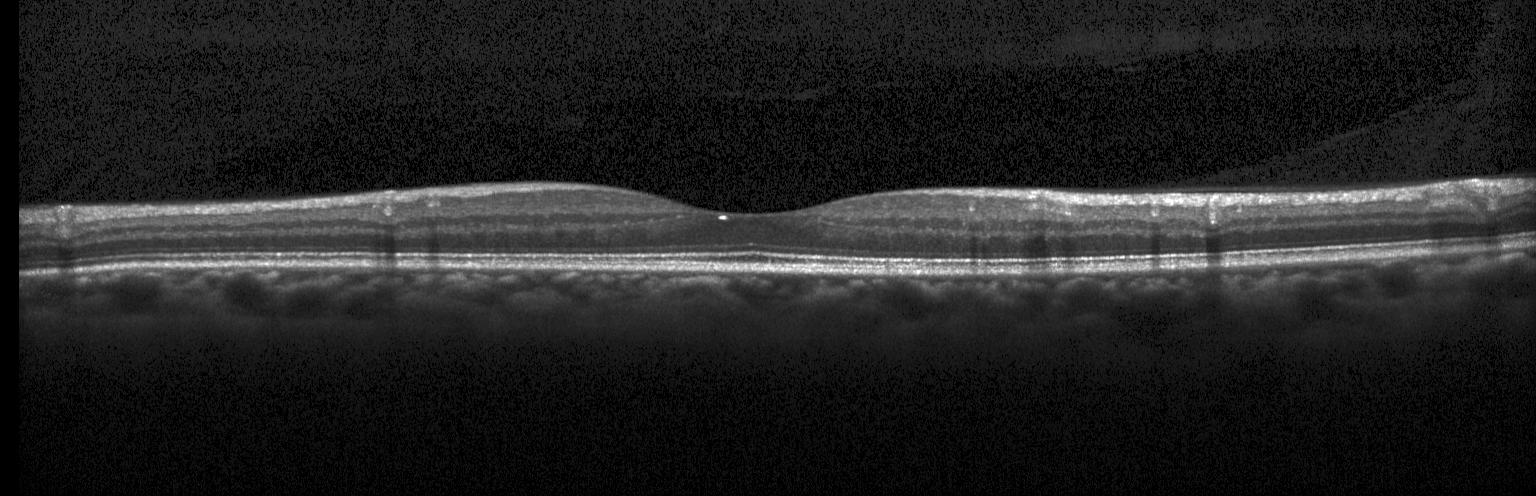
Spectral-domain OCT, optical coherence tomography scan, centered on the fovea, acquired on a Heidelberg Spectralis.
Dx: no evidence of CNV, DME, or drusen.